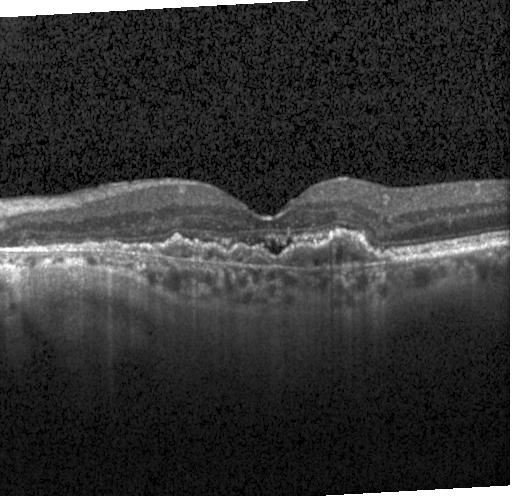
Acquired on a Heidelberg Spectralis · spectral-domain optical coherence tomography · retinal OCT cross-section.
A choroidal neovascular membrane.